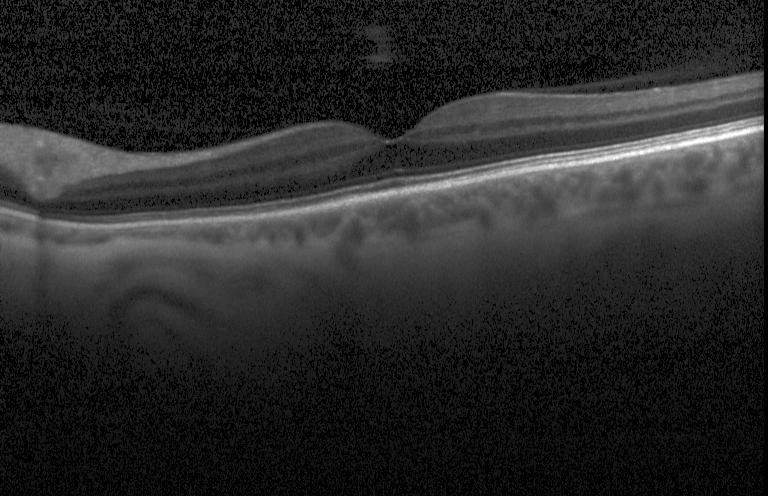 Acquired on a Heidelberg Spectralis. Spectral-domain optical coherence tomography. Fovea-centered. Optical coherence tomography B-scan
Finding: no evidence of choroidal neovascularization, diabetic macular edema, or drusen.